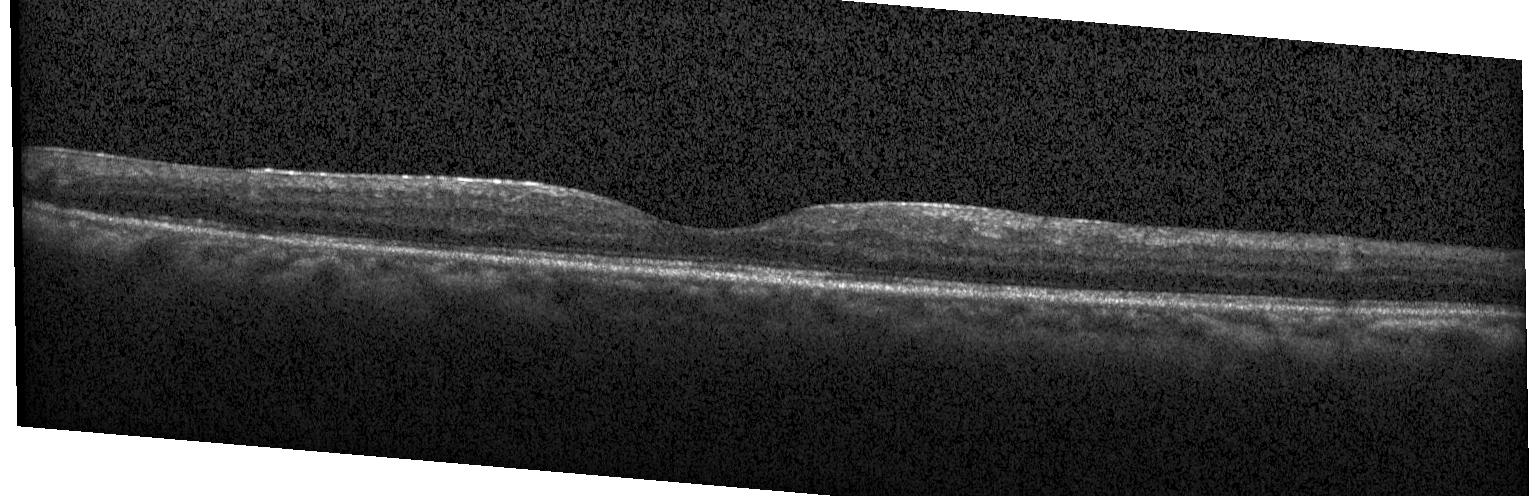

OCT line scan.
OCT finding: no evidence of choroidal neovascularization, diabetic macular edema, or drusen.